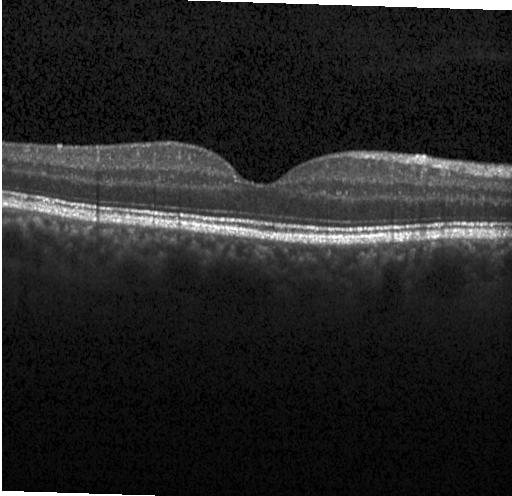
Assessment: no CNV, DME, or drusen.